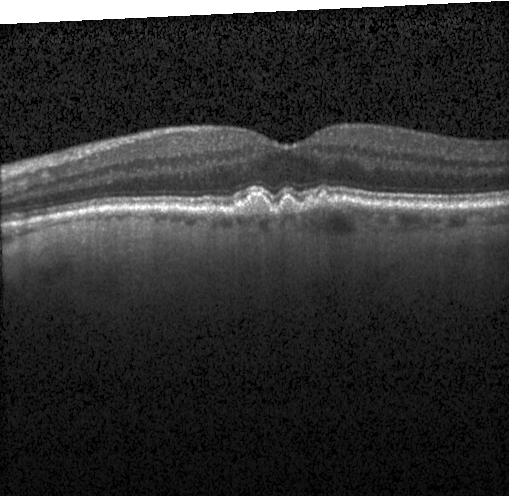

Optical coherence tomography B-scan. This B-scan demonstrates sub-RPE drusenoid deposits.